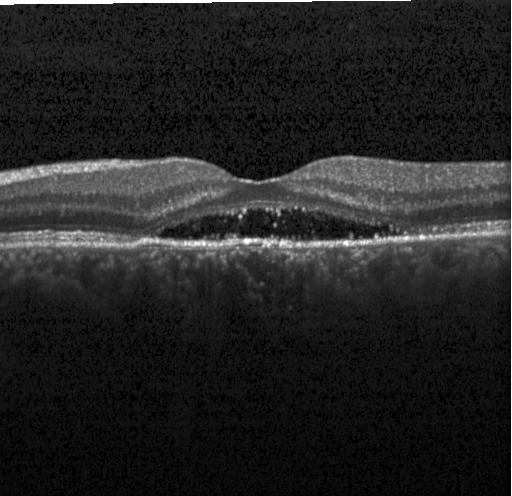

Finding: a choroidal neovascular membrane.